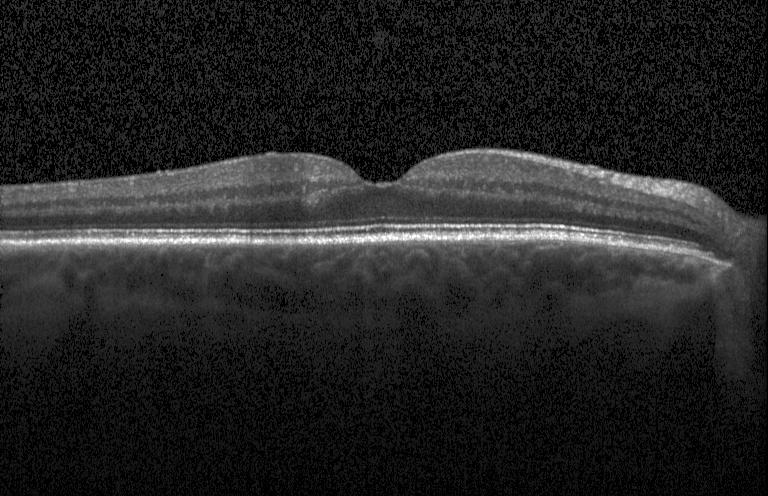

OCT line scan · centered on the fovea.
This B-scan demonstrates no choroidal neovascularization, no diabetic macular edema, and no drusen.